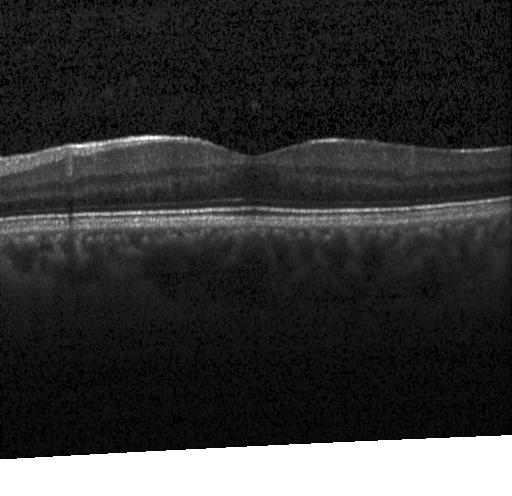 Finding: neither choroidal neovascularization, diabetic macular edema, nor drusen.